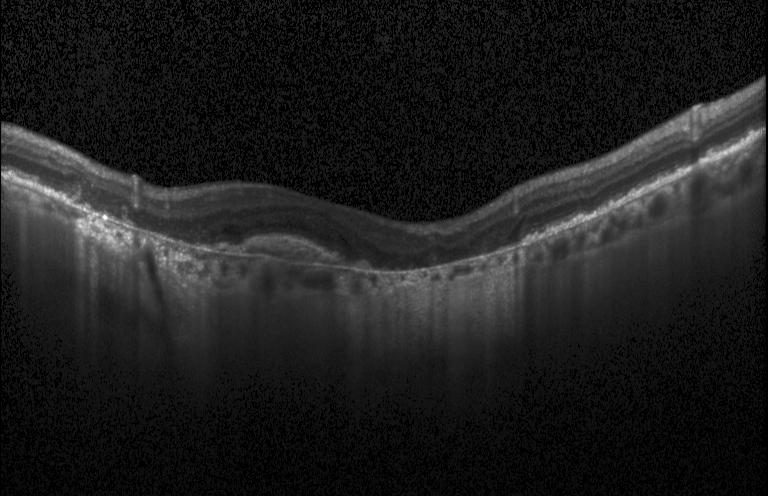 OCT line scan; SD-OCT; fovea-centered.
Finding: a choroidal neovascular membrane.